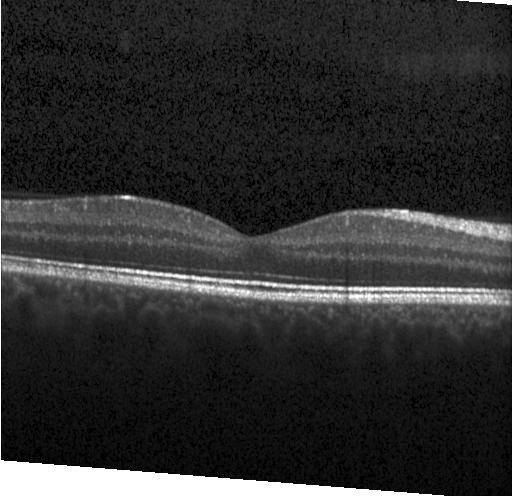 The scan shows no evidence of CNV, DME, or drusen.